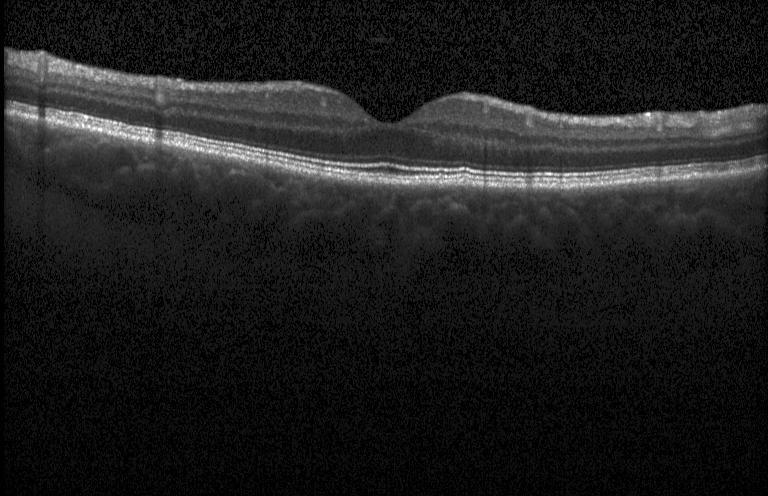 Through the macula, retinal OCT B-scan, spectral-domain OCT
Assessment: no choroidal neovascularization, no diabetic macular edema, and no drusen.